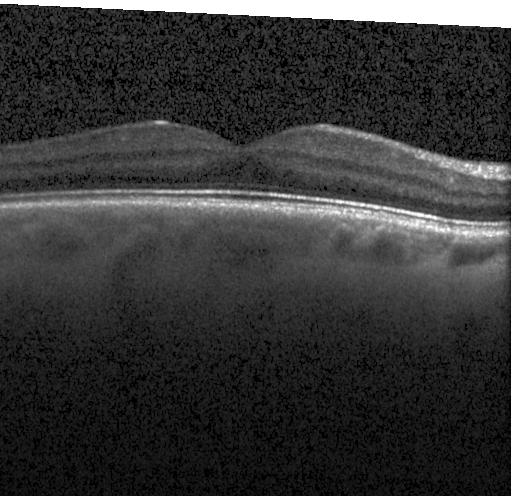 Retinal OCT cross-section — Diagnosis: no evidence of CNV, DME, or drusen.